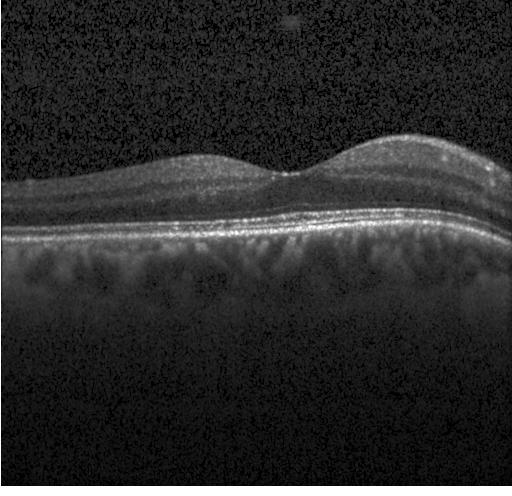 Optical coherence tomography B-scan. SD-OCT. Finding: no choroidal neovascularization, diabetic macular edema, or drusen.